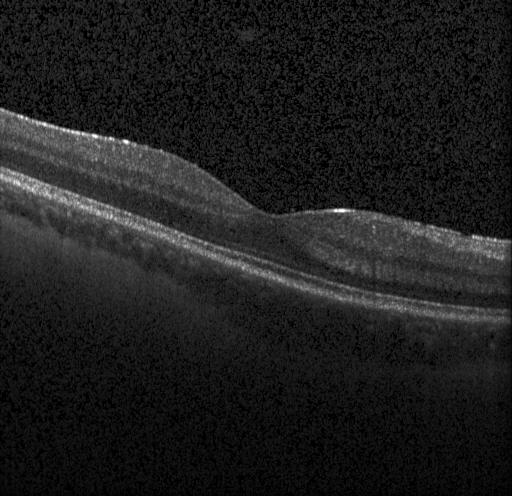
Heidelberg Spectralis · optical coherence tomography B-scan — Dx: no evidence of CNV, DME, or drusen.